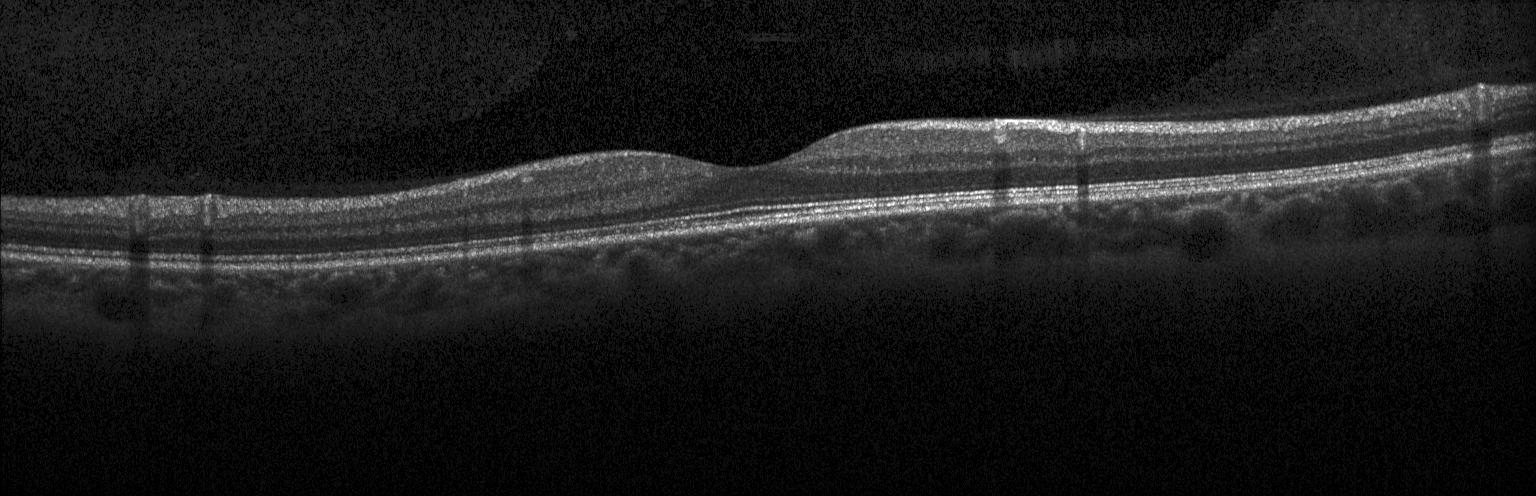
Instrument: Heidelberg Spectralis. Optical coherence tomography scan. SD-OCT.
Impression: neither CNV, DME, nor drusen.